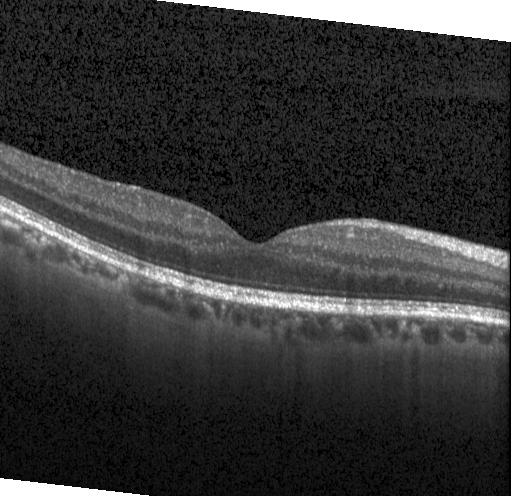
Heidelberg Spectralis. OCT B-scan.
No choroidal neovascularization, no diabetic macular edema, and no drusen.